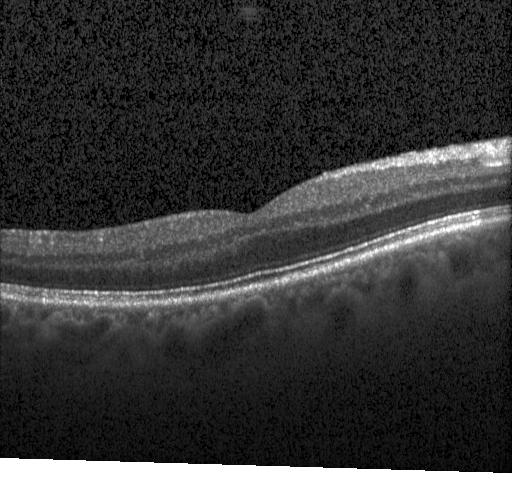 Macular scan · retinal OCT cross-section · spectral-domain OCT — Macular OCT: no choroidal neovascularization, no diabetic macular edema, and no drusen.